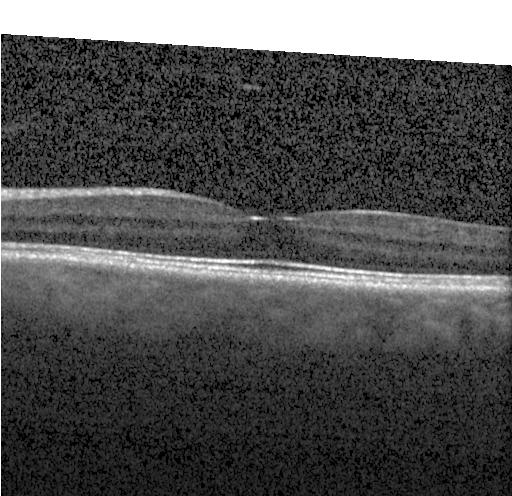 Retinal OCT cross-section showing no CNV, DME, or drusen.